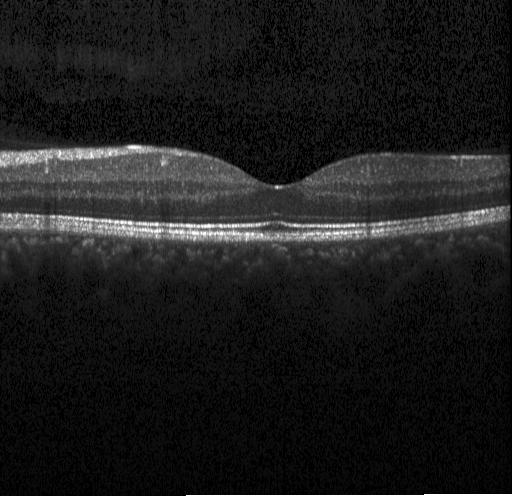 Macular OCT: no evidence of CNV, DME, or drusen.